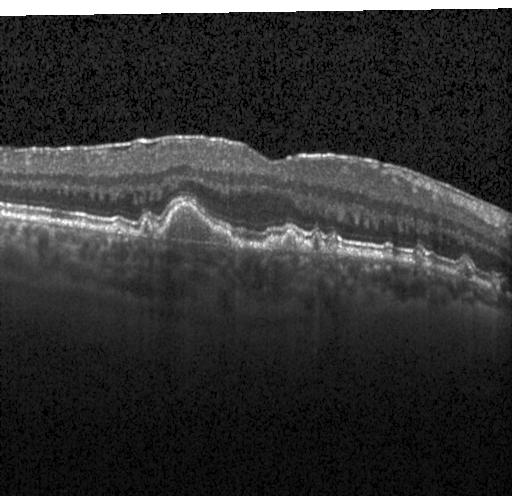 CNV.